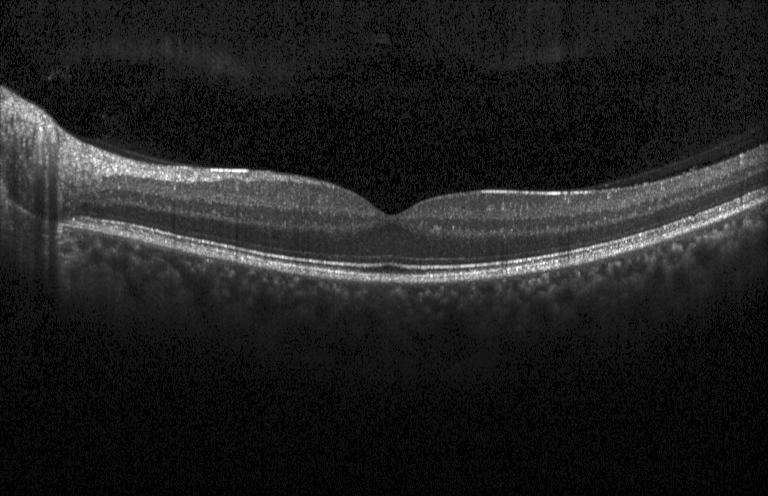 Spectral-domain optical coherence tomography · optical coherence tomography scan · fovea-centered — Finding: no choroidal neovascularization, diabetic macular edema, or drusen.